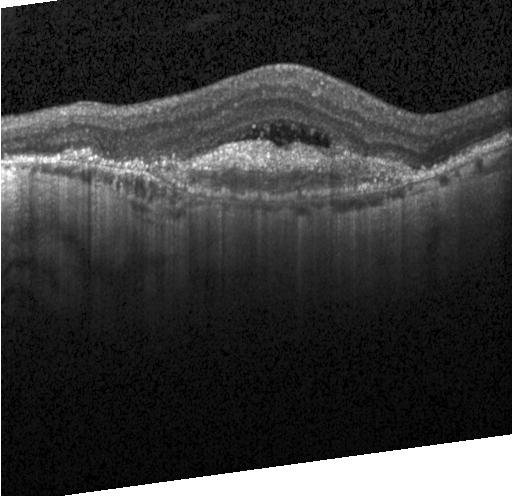
Diagnosis: a choroidal neovascular membrane.